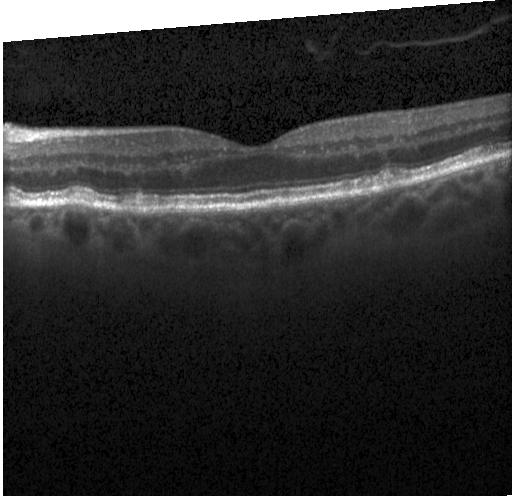
OCT finding: multiple drusen.